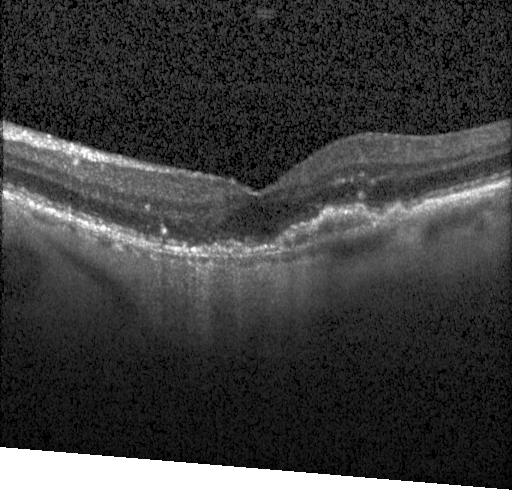 OCT B-scan. Dx: a choroidal neovascular membrane.